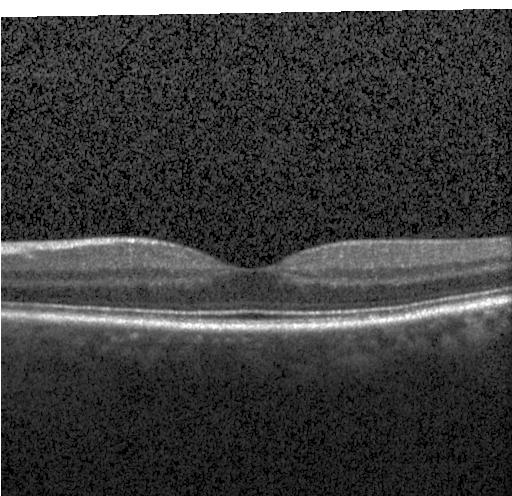 Fovea-centered; OCT line scan; Heidelberg Spectralis OCT system; spectral-domain optical coherence tomography.
This B-scan demonstrates no choroidal neovascularization, diabetic macular edema, or drusen.